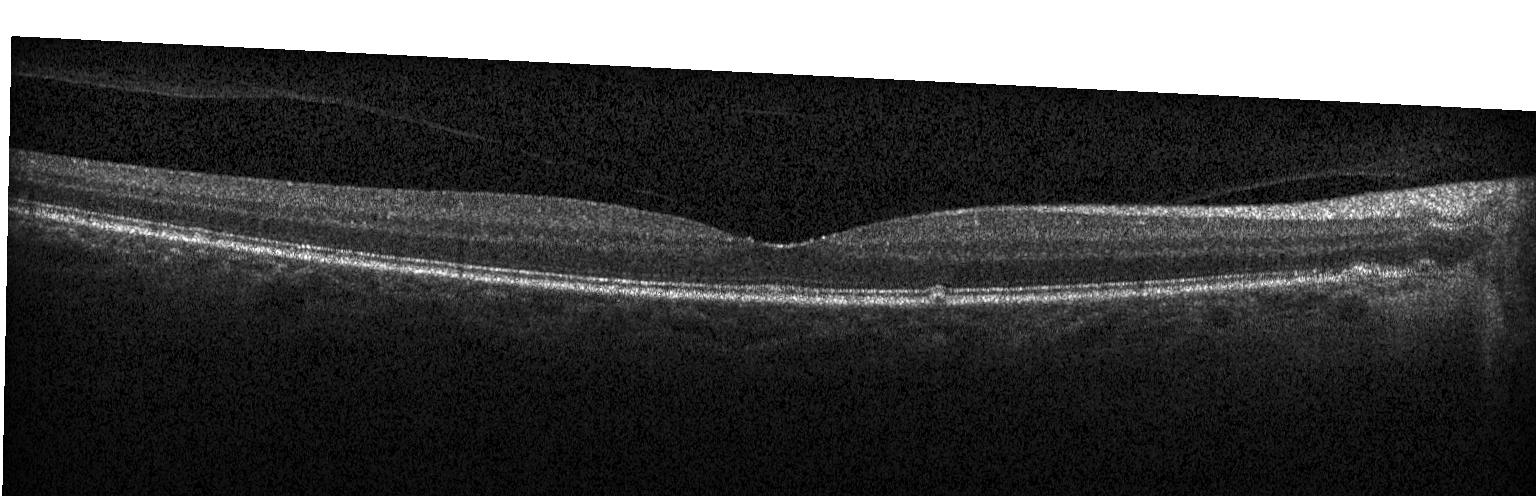 SD-OCT · OCT B-scan · through the macula.
Multiple drusen.